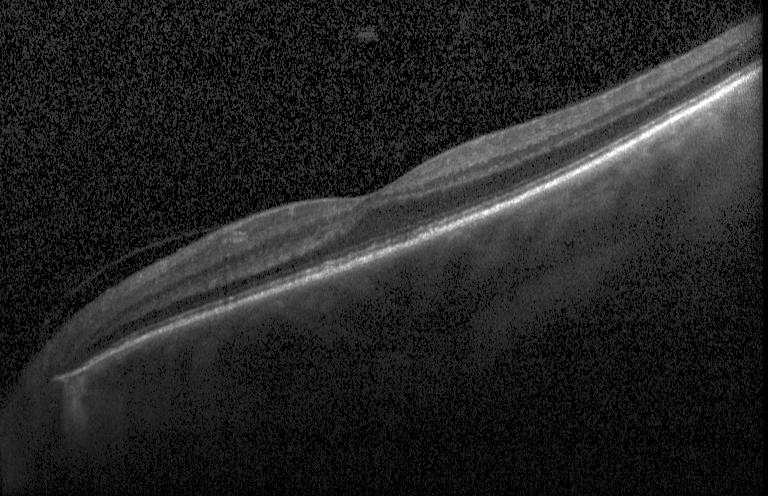 Horizontal scan through the fovea · retinal OCT cross-section.
Impression: no choroidal neovascularization, no diabetic macular edema, and no drusen.